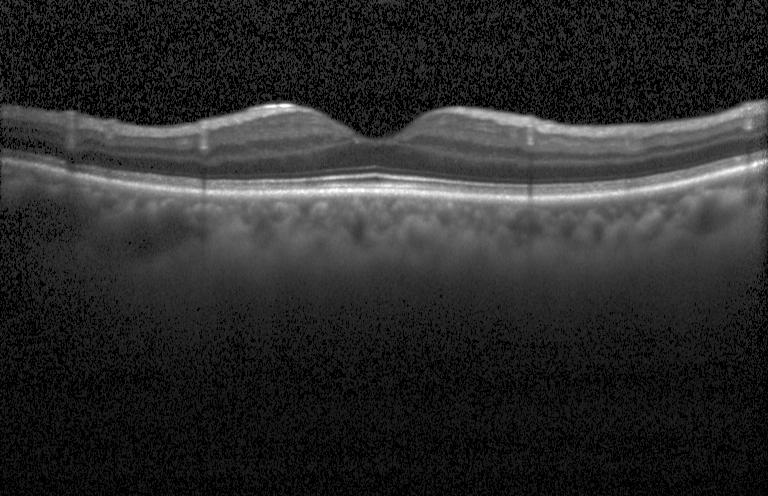
Optical coherence tomography scan, Heidelberg Spectralis OCT system, spectral-domain OCT.
Impression: neither choroidal neovascularization, diabetic macular edema, nor drusen.